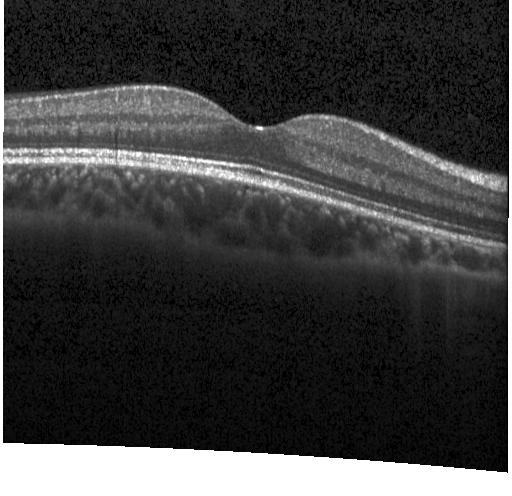

Through the macula; optical coherence tomography scan. Diagnosis: no evidence of choroidal neovascularization, diabetic macular edema, or drusen.